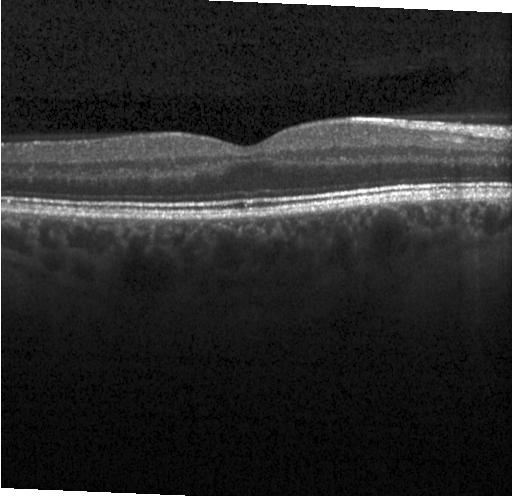

Optical coherence tomography B-scan. Horizontal scan through the fovea. Dx: no evidence of CNV, DME, or drusen.